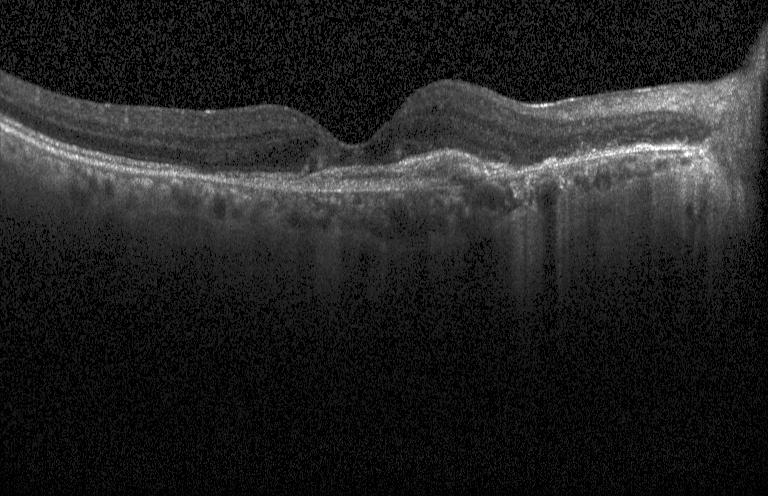

Retinal OCT cross-section
Impression: choroidal neovascularization (CNV).